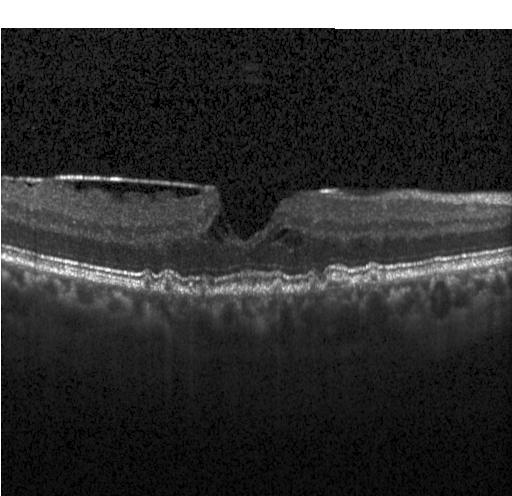
Spectral-domain optical coherence tomography; Heidelberg Spectralis; OCT line scan — Impression: drusen.